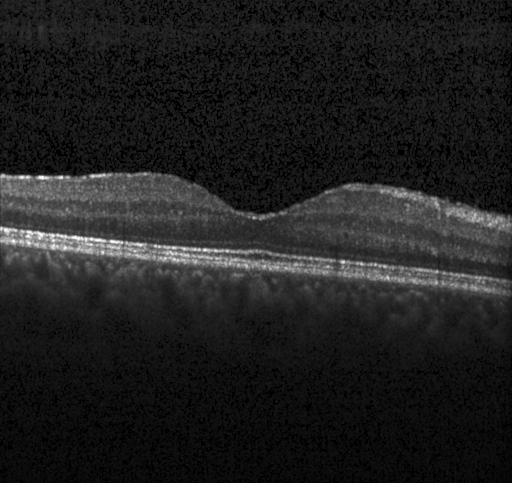
The scan shows neither choroidal neovascularization, diabetic macular edema, nor drusen.